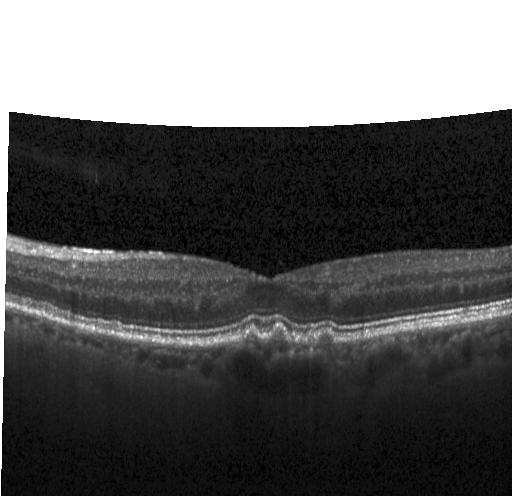 Spectral-domain OCT B-scan: drusen.